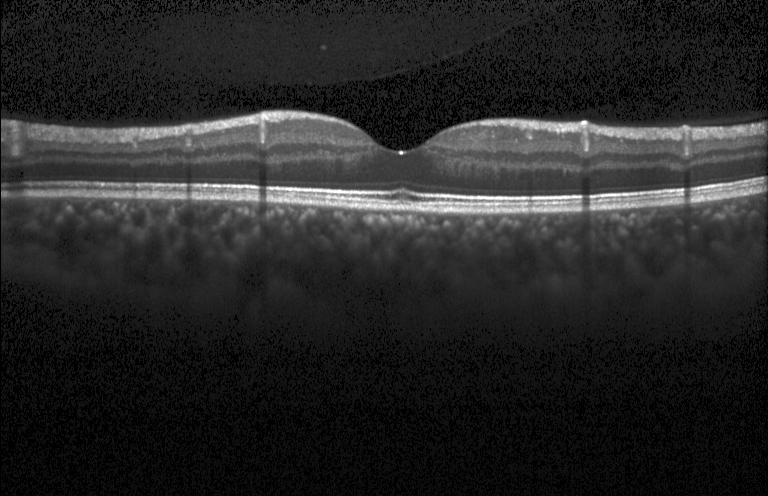 Impression: no CNV, no DME, and no drusen.